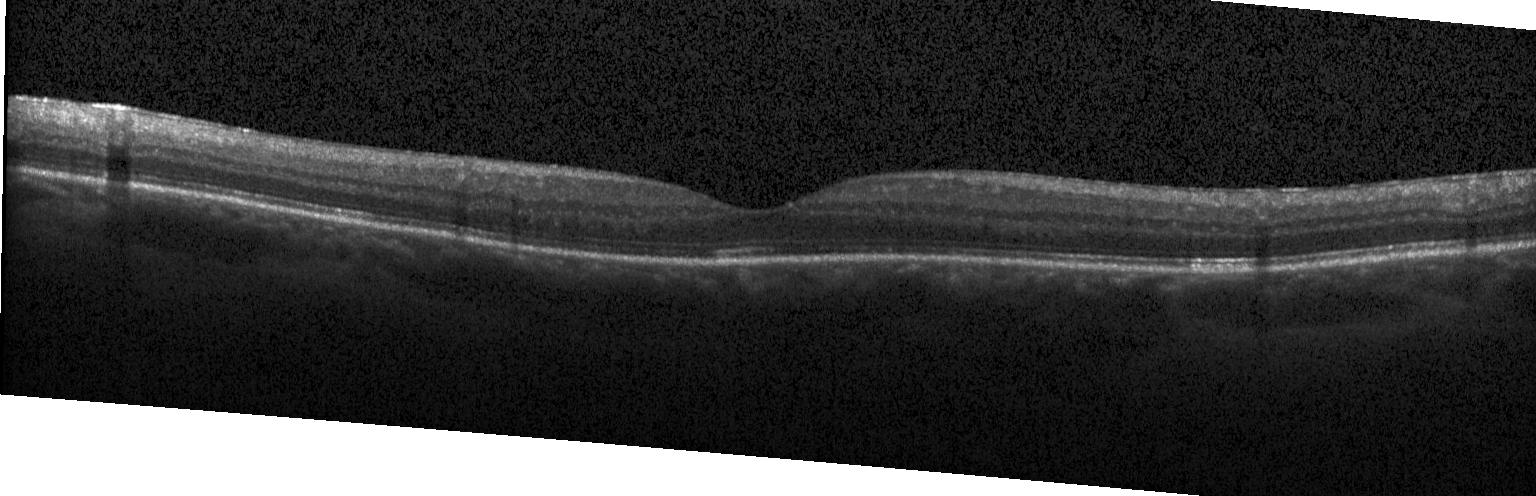
Retinal OCT B-scan. Assessment: no CNV, no DME, and no drusen.